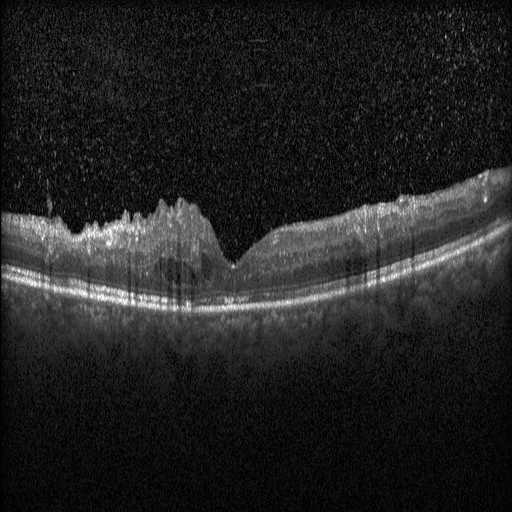
Retinal OCT cross-section.
Finding: diabetic macular edema (DME).